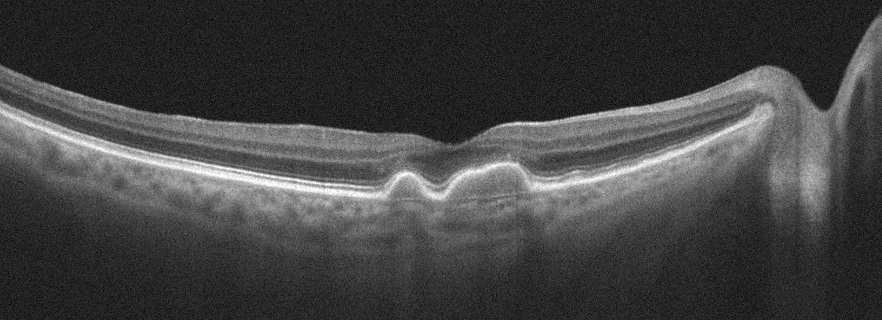 Optovue Avanti RTVue XR · fovea-centered · retinal OCT cross-section. OCT finding: age-related macular degeneration.